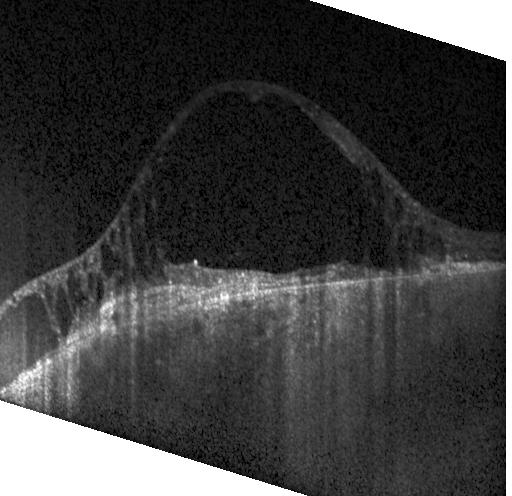

Centered on the fovea; Heidelberg Spectralis OCT system; retinal OCT B-scan. Macular OCT: a choroidal neovascular membrane.